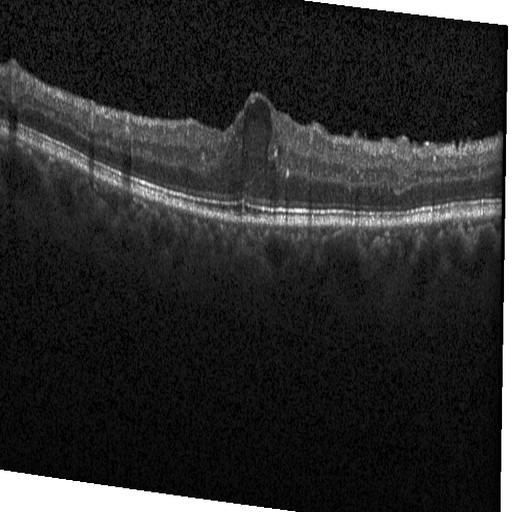 Acquired on a Heidelberg Spectralis. Horizontal scan through the fovea. Spectral-domain optical coherence tomography. Retinal OCT B-scan. Diagnosis: diabetic macular edema.